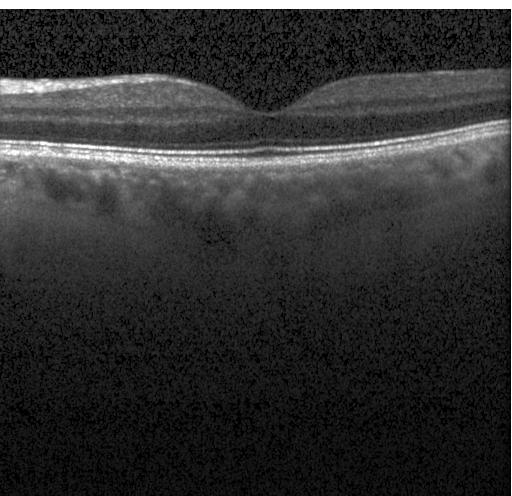
Retinal OCT B-scan; spectral-domain OCT; fovea-centered; acquired on a Heidelberg Spectralis. Impression: no evidence of CNV, DME, or drusen.